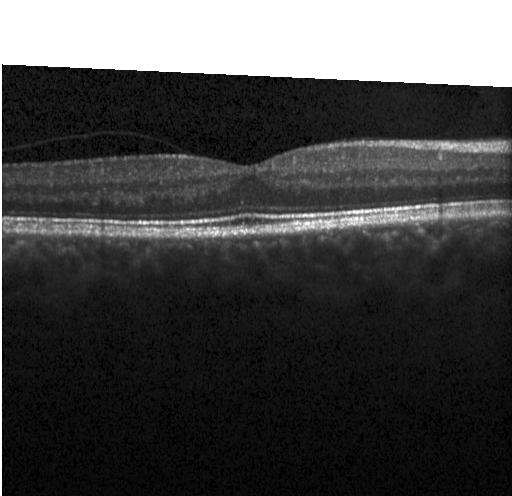

Optical coherence tomography B-scan; Heidelberg Spectralis OCT system — Finding: no choroidal neovascularization, no diabetic macular edema, and no drusen.